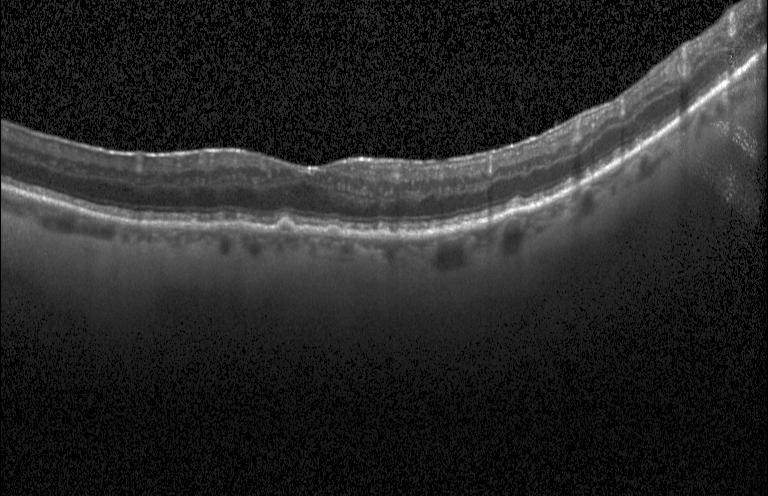
OCT line scan, Heidelberg Spectralis, spectral-domain optical coherence tomography
Finding: drusen.